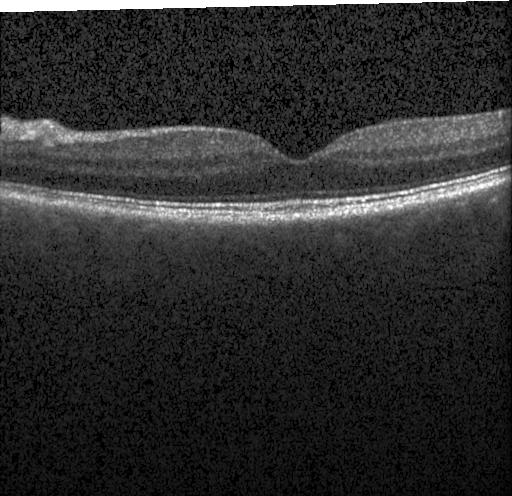 Heidelberg Spectralis OCT system; OCT B-scan.
Assessment: neither choroidal neovascularization, diabetic macular edema, nor drusen.